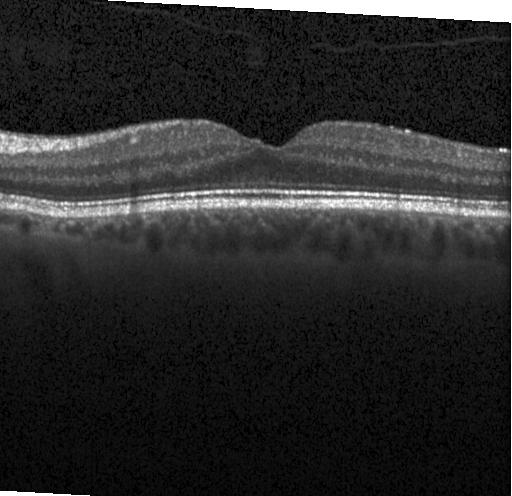

Optical coherence tomography scan
Dx: no choroidal neovascularization, diabetic macular edema, or drusen.